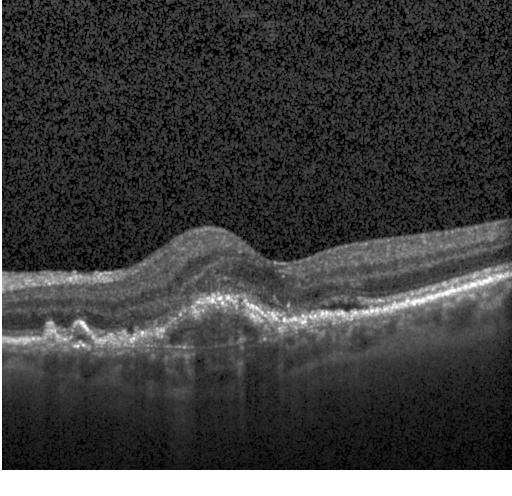

Impression: CNV.